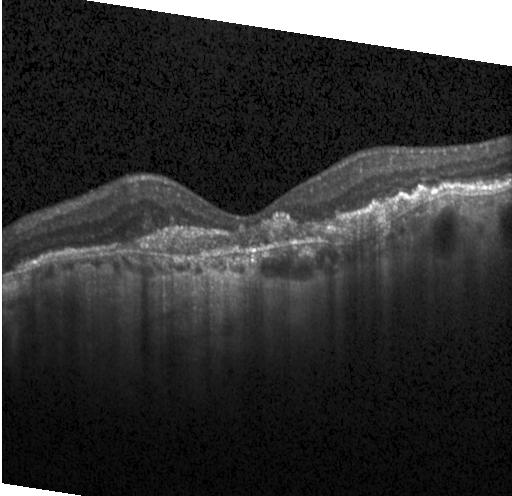 Diagnosis: a choroidal neovascular membrane.